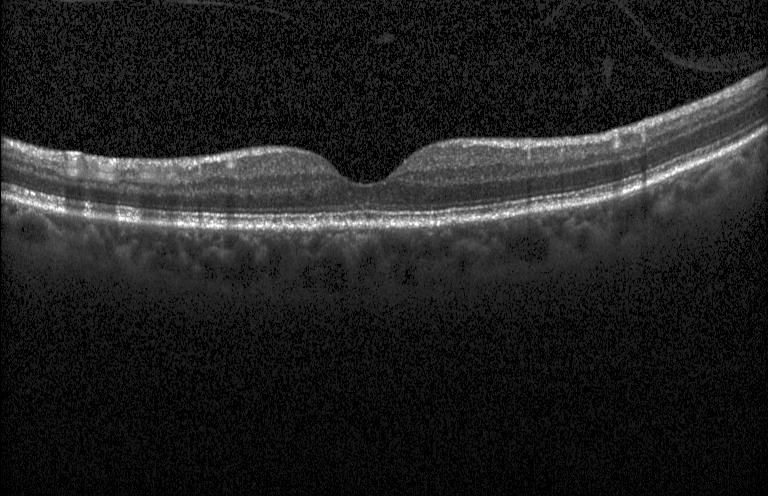
Spectral-domain optical coherence tomography; OCT line scan; fovea-centered
OCT finding: no choroidal neovascularization, no diabetic macular edema, and no drusen.